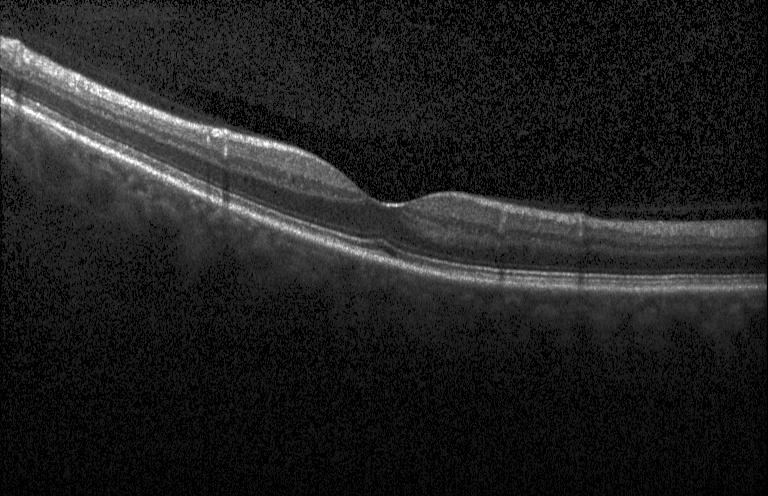 Macular OCT demonstrating no choroidal neovascularization, diabetic macular edema, or drusen.